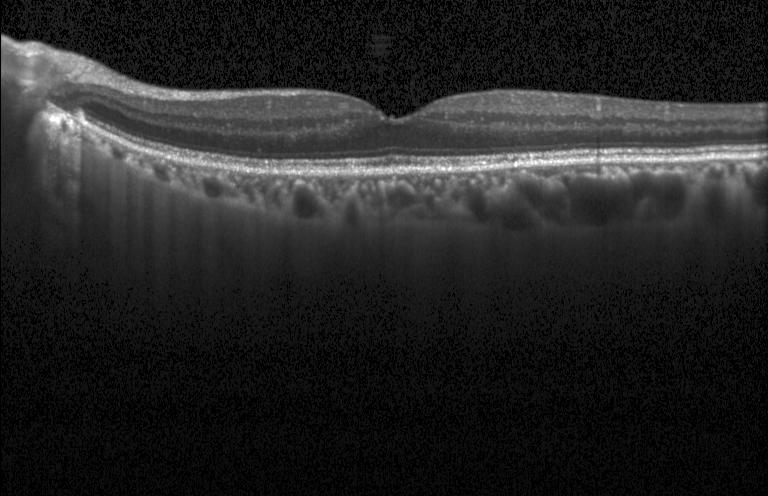
OCT B-scan
Assessment: neither CNV, DME, nor drusen.